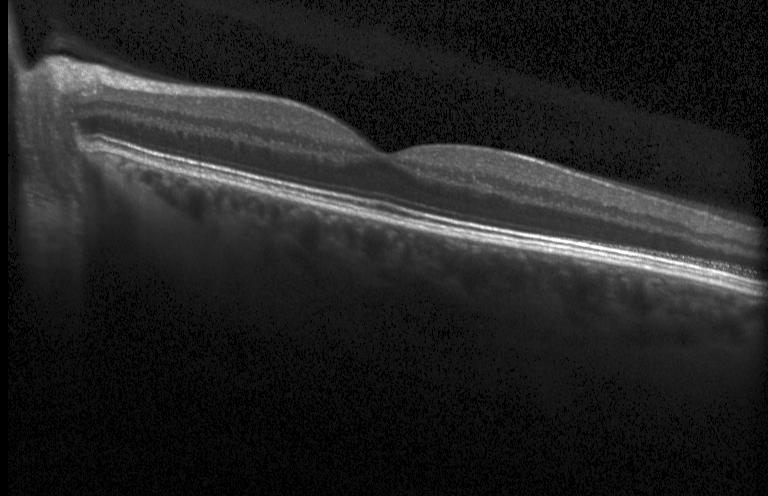
Through the macula · spectral-domain optical coherence tomography · optical coherence tomography scan · instrument: Heidelberg Spectralis. Diagnosis: no evidence of CNV, DME, or drusen.